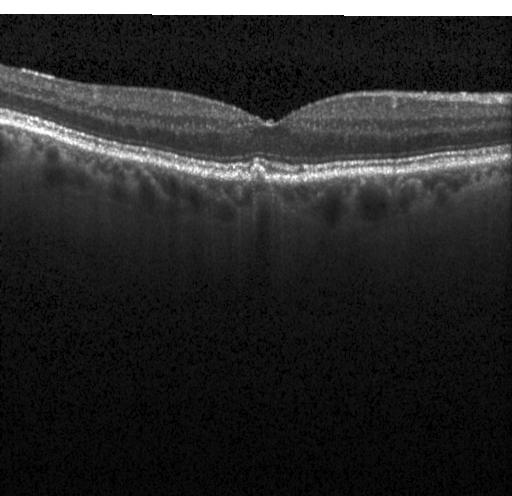 Macular scan. Optical coherence tomography B-scan. Finding: sub-RPE drusenoid deposits.